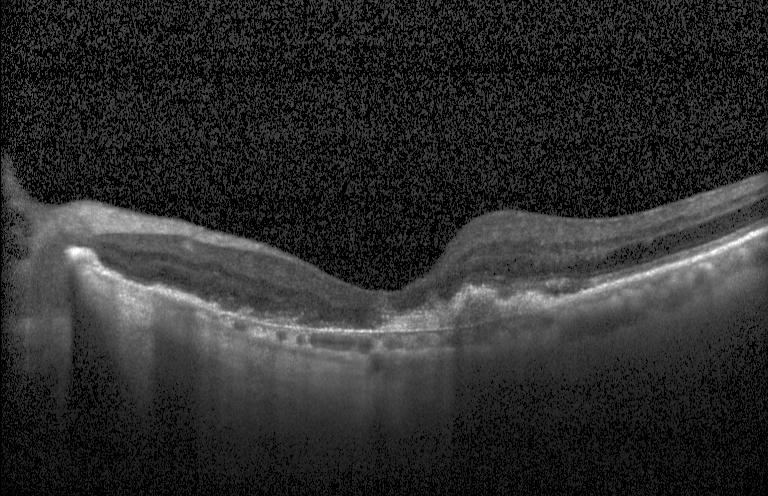

OCT finding: a choroidal neovascular membrane.